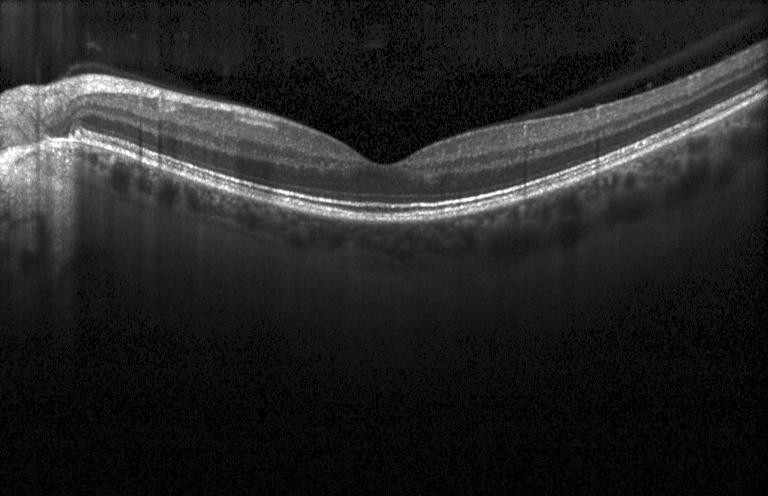

Spectral-domain OCT B-scan: no evidence of CNV, DME, or drusen.